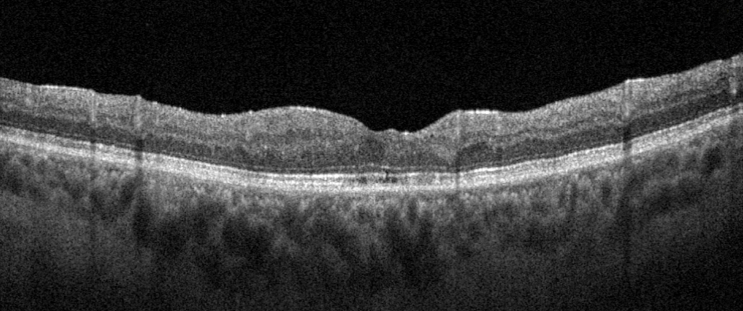

Instrument: Optovue Avanti RTVue XR. Optical coherence tomography scan
Diabetic macular edema (DME).